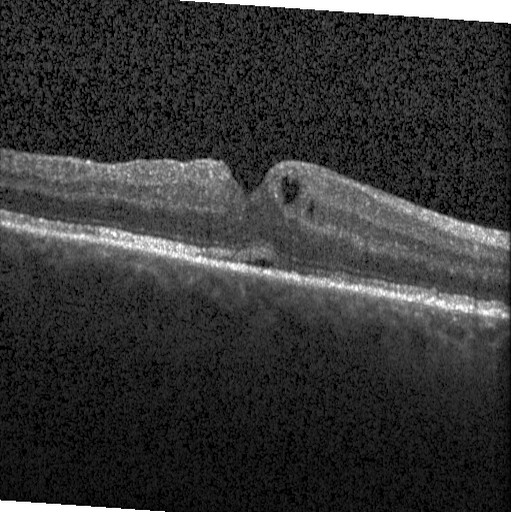

This B-scan demonstrates diabetic macular edema (DME).